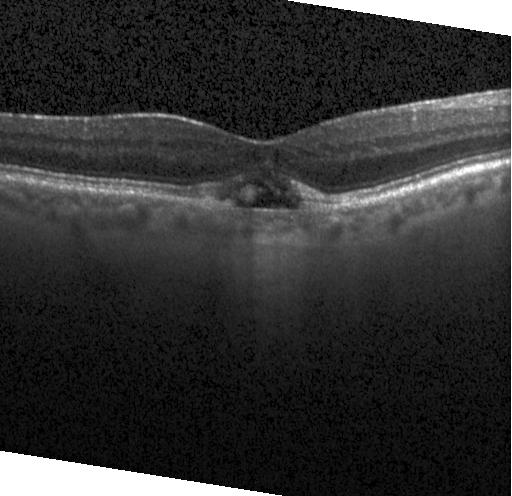 This B-scan demonstrates a choroidal neovascular membrane.